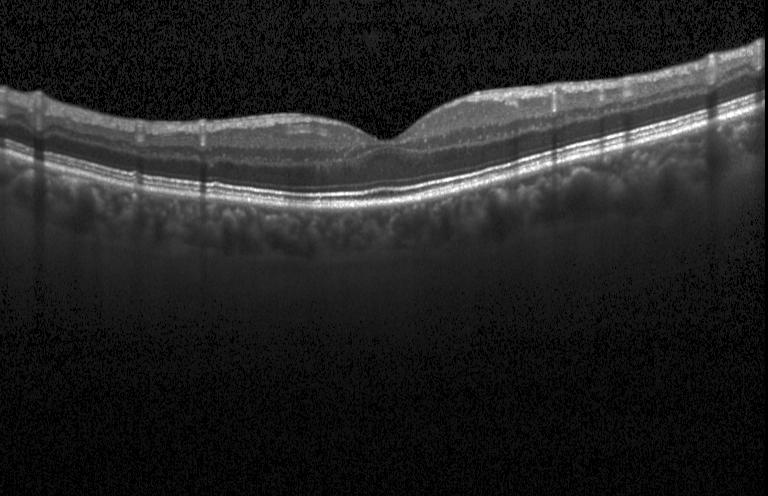
Macular OCT demonstrating neither choroidal neovascularization, diabetic macular edema, nor drusen.